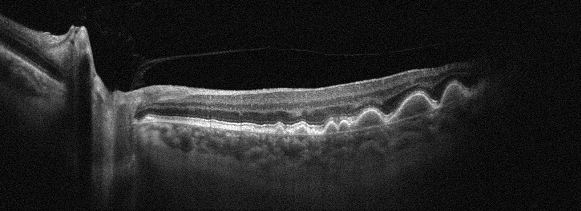 Macular OCT: age-related macular degeneration (AMD).